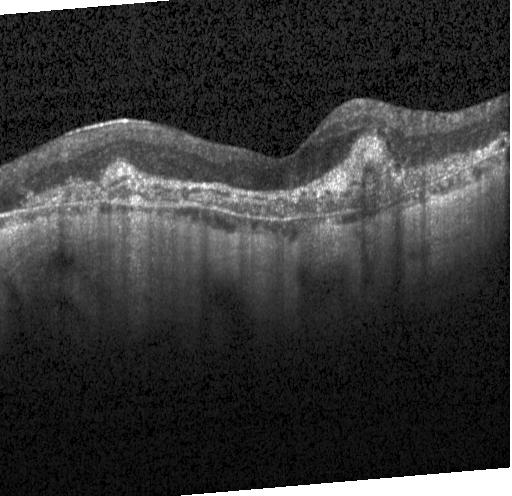 Diagnosis: choroidal neovascularization.